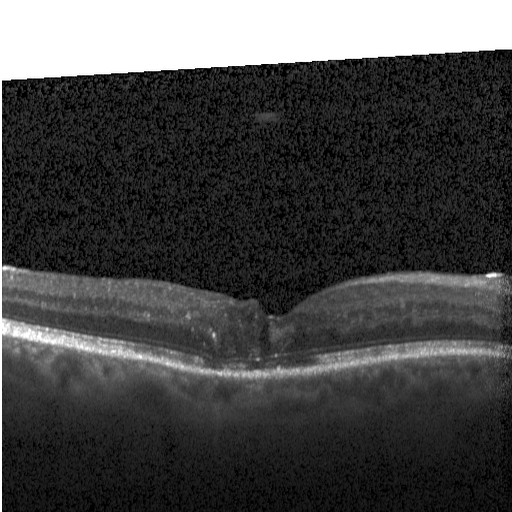
Spectral-domain OCT. Heidelberg Spectralis OCT system. Macular scan. Optical coherence tomography B-scan — Diagnosis: diabetic macular edema (DME).